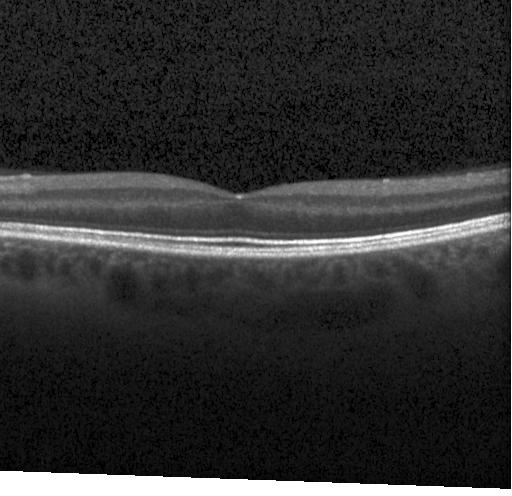

Horizontal scan through the fovea; retinal OCT cross-section.
This B-scan demonstrates neither choroidal neovascularization, diabetic macular edema, nor drusen.